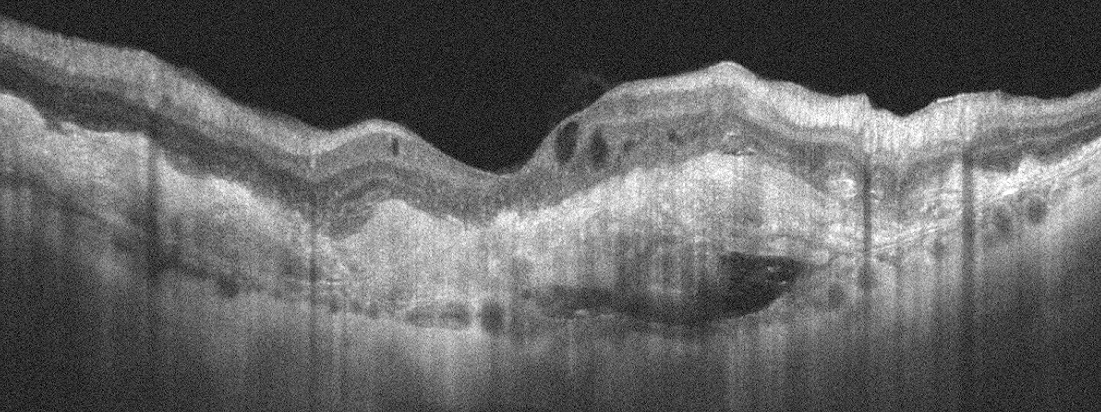

This B-scan demonstrates age-related macular degeneration (AMD).